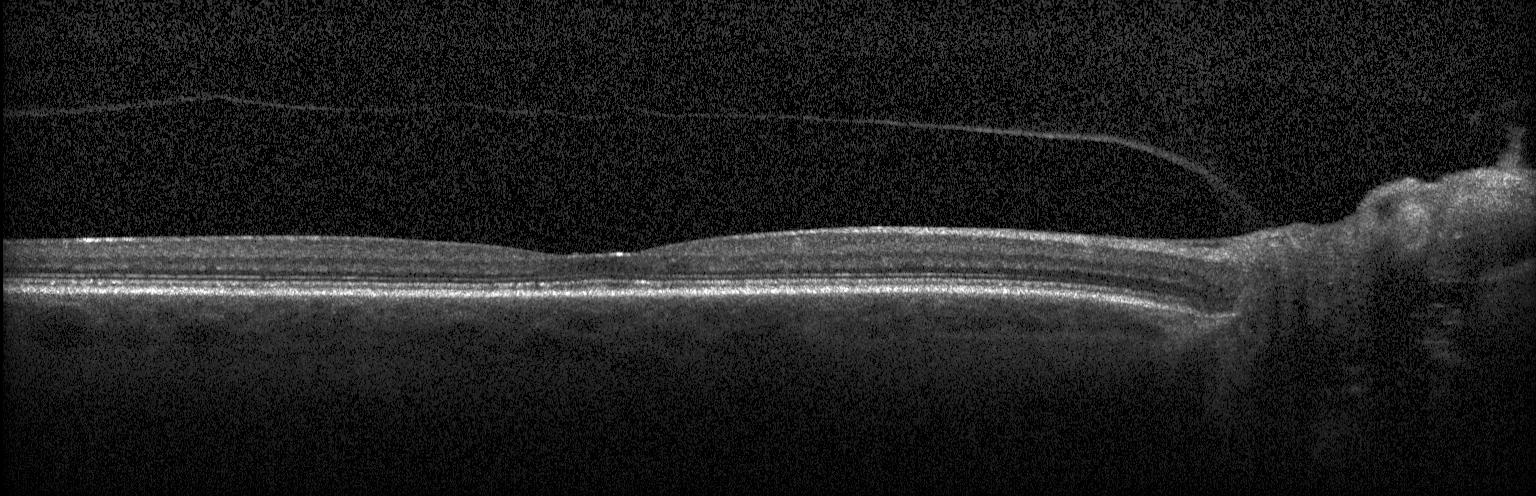 Retinal OCT cross-section — Impression: no CNV, no DME, and no drusen.